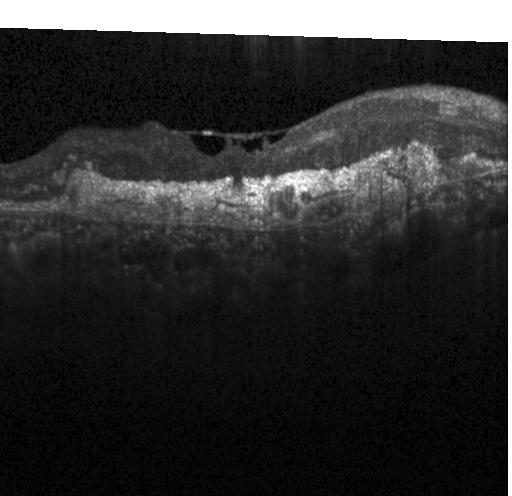

Heidelberg Spectralis, retinal OCT B-scan, SD-OCT.
Impression: a choroidal neovascular membrane.